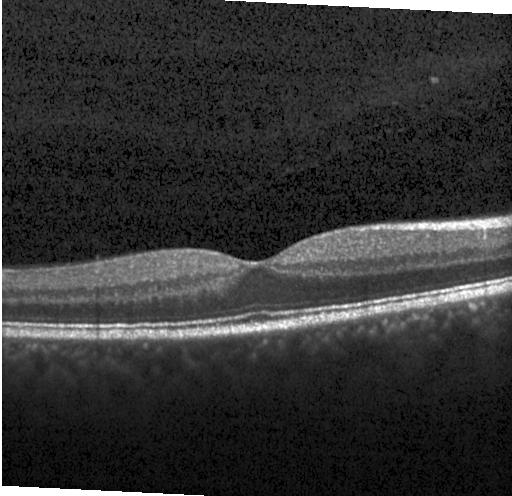
Acquired on a Heidelberg Spectralis. OCT line scan. Macular scan.
Macular OCT: neither CNV, DME, nor drusen.